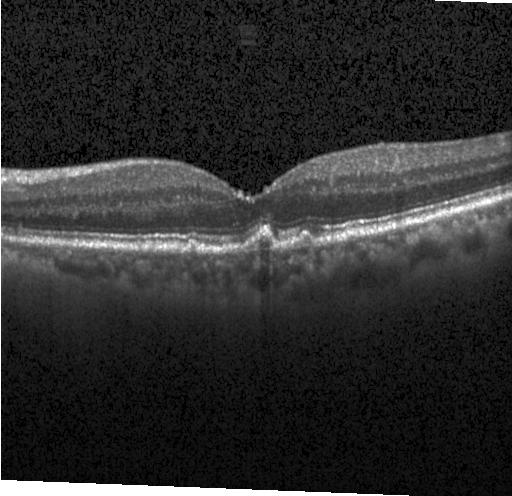 Optical coherence tomography B-scan, Heidelberg Spectralis OCT system, spectral-domain optical coherence tomography, horizontal scan through the fovea. Diagnosis: multiple drusen.